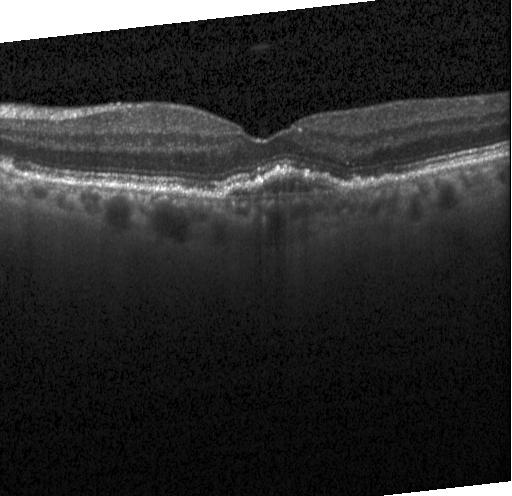
OCT B-scan; spectral-domain optical coherence tomography; Heidelberg Spectralis.
Diagnosis: a choroidal neovascular membrane.